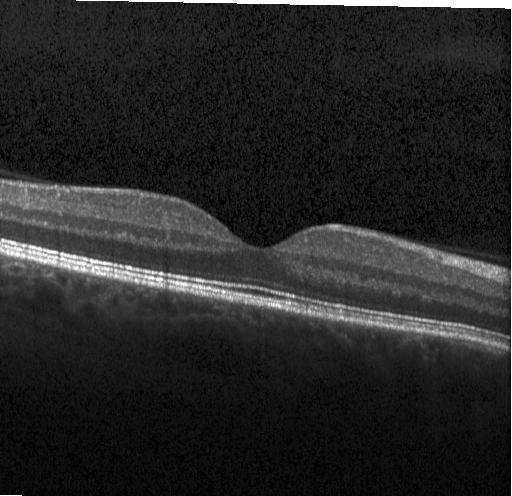

Spectral-domain optical coherence tomography, retinal OCT cross-section, Heidelberg Spectralis, centered on the fovea. Macular OCT: neither choroidal neovascularization, diabetic macular edema, nor drusen.